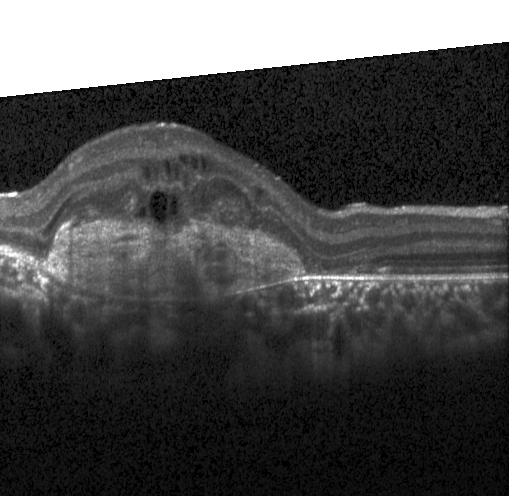

Impression: a choroidal neovascular membrane.